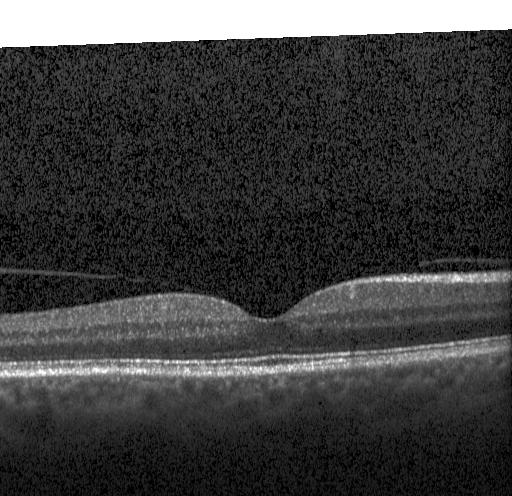 Retinal OCT B-scan, SD-OCT, instrument: Heidelberg Spectralis, through the macula — OCT finding: neither choroidal neovascularization, diabetic macular edema, nor drusen.